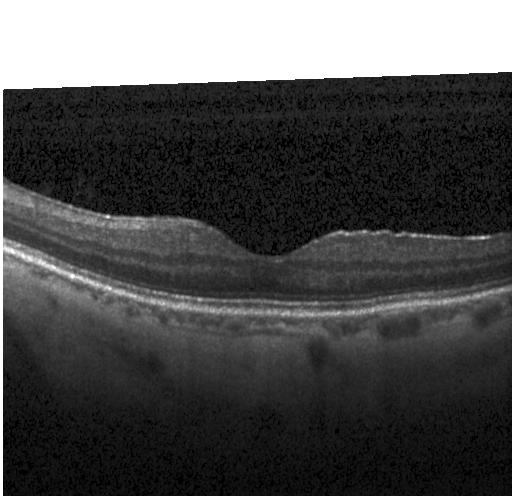 Dx: no evidence of choroidal neovascularization, diabetic macular edema, or drusen.